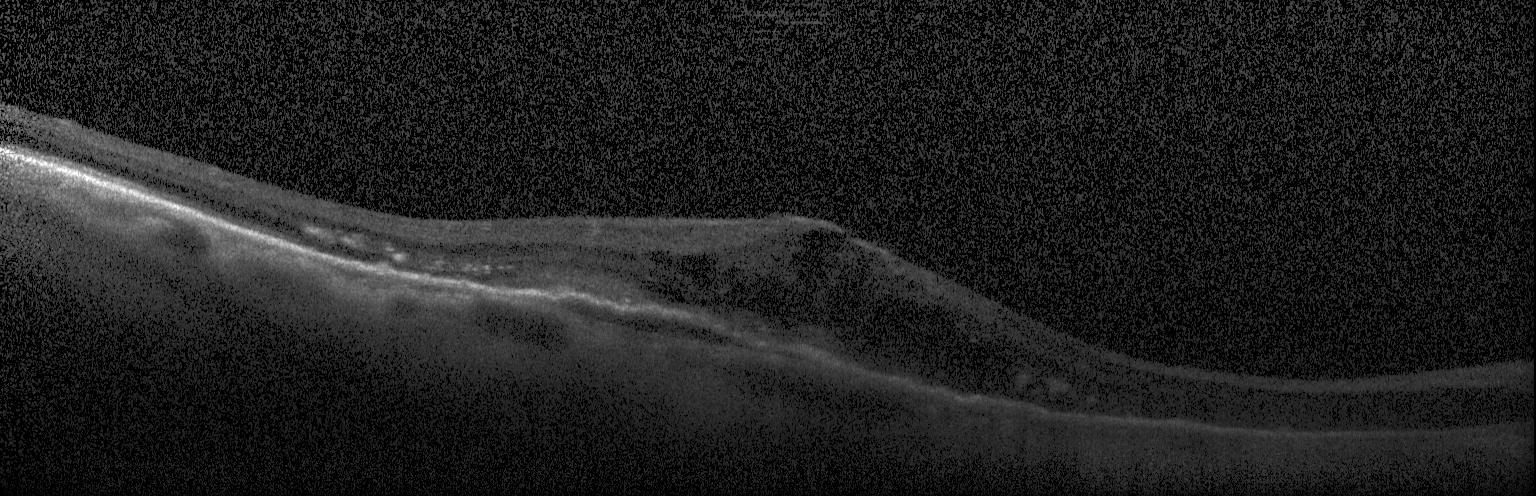

Diagnosis: choroidal neovascularization.